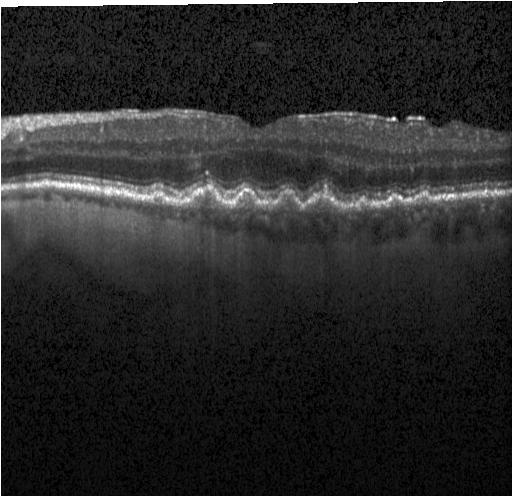
OCT line scan.
Finding: sub-RPE drusenoid deposits.